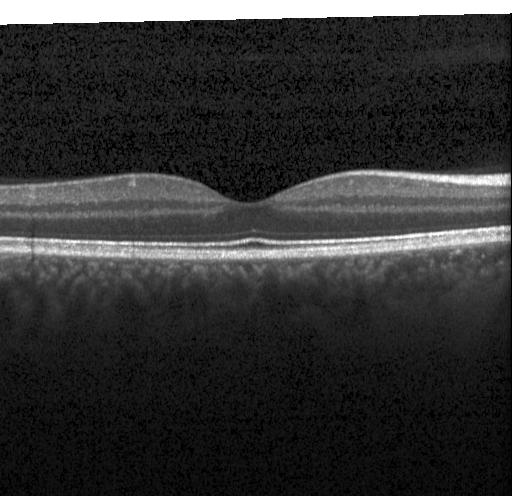
SD-OCT; retinal OCT B-scan; horizontal scan through the fovea — Assessment: no evidence of CNV, DME, or drusen.